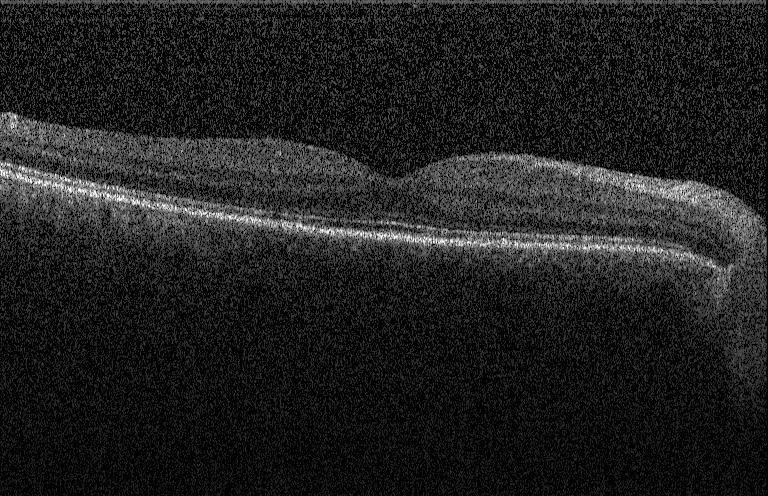

Impression: neither CNV, DME, nor drusen.